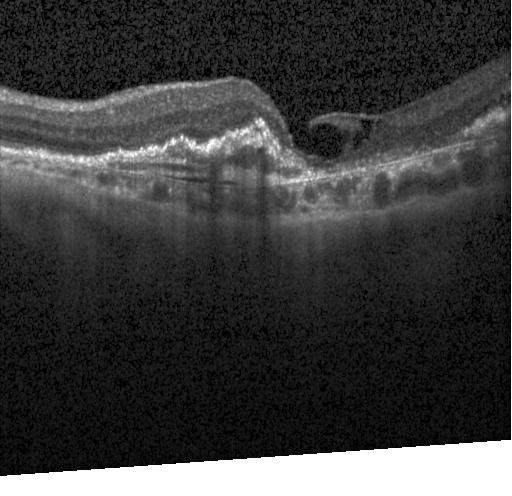
Spectral-domain OCT B-scan: CNV.